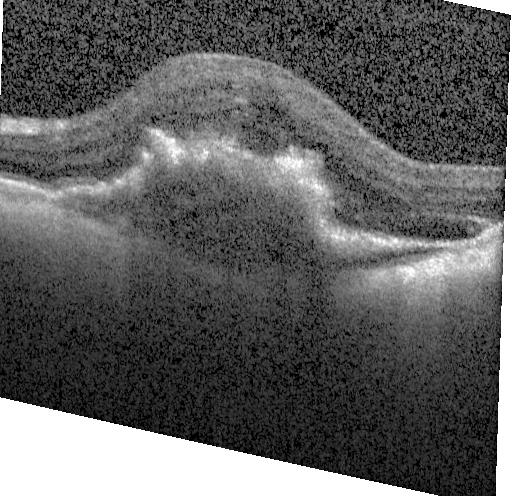 Impression: choroidal neovascularization.